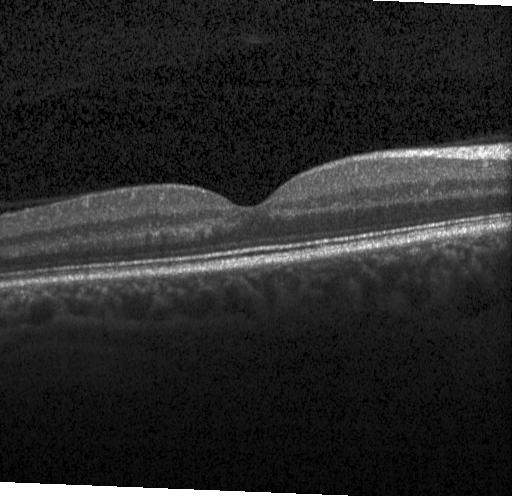

Diagnosis: neither choroidal neovascularization, diabetic macular edema, nor drusen.